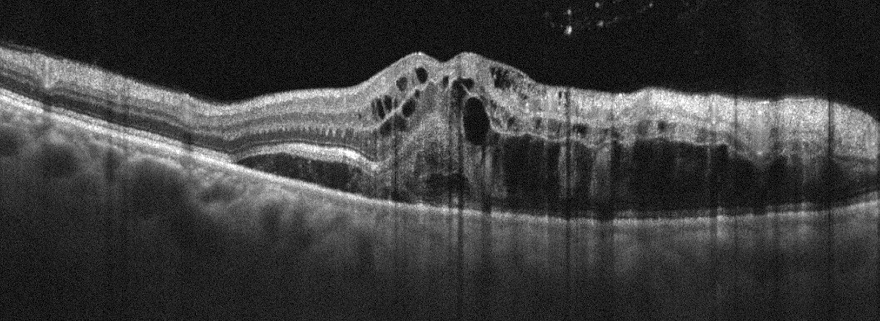 OCT B-scan; Optovue Avanti RTVue XR — Assessment: retinal vein occlusion (RVO).